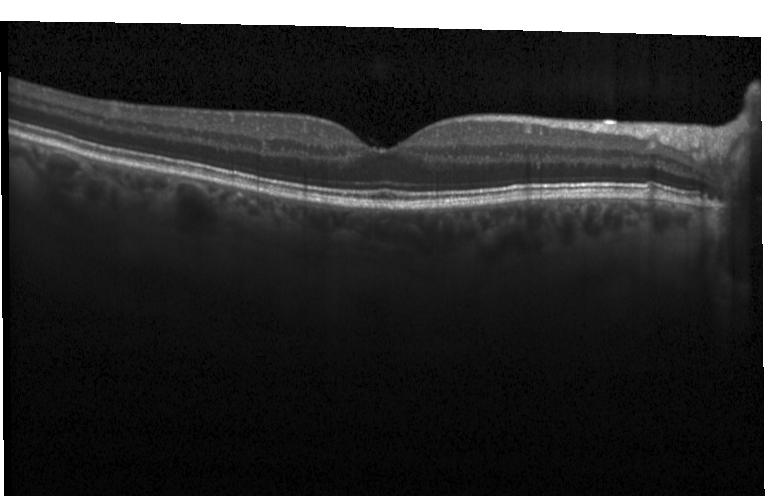
OCT line scan · centered on the fovea · instrument: Heidelberg Spectralis · SD-OCT. Impression: neither CNV, DME, nor drusen.